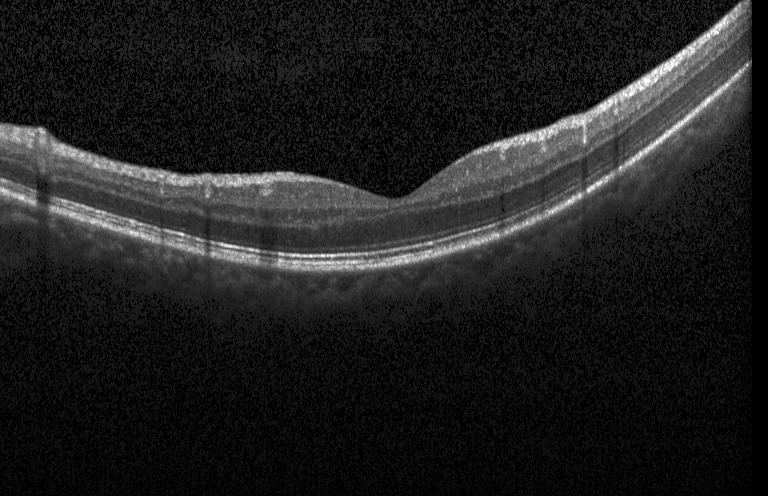
Assessment: no CNV, no DME, and no drusen.